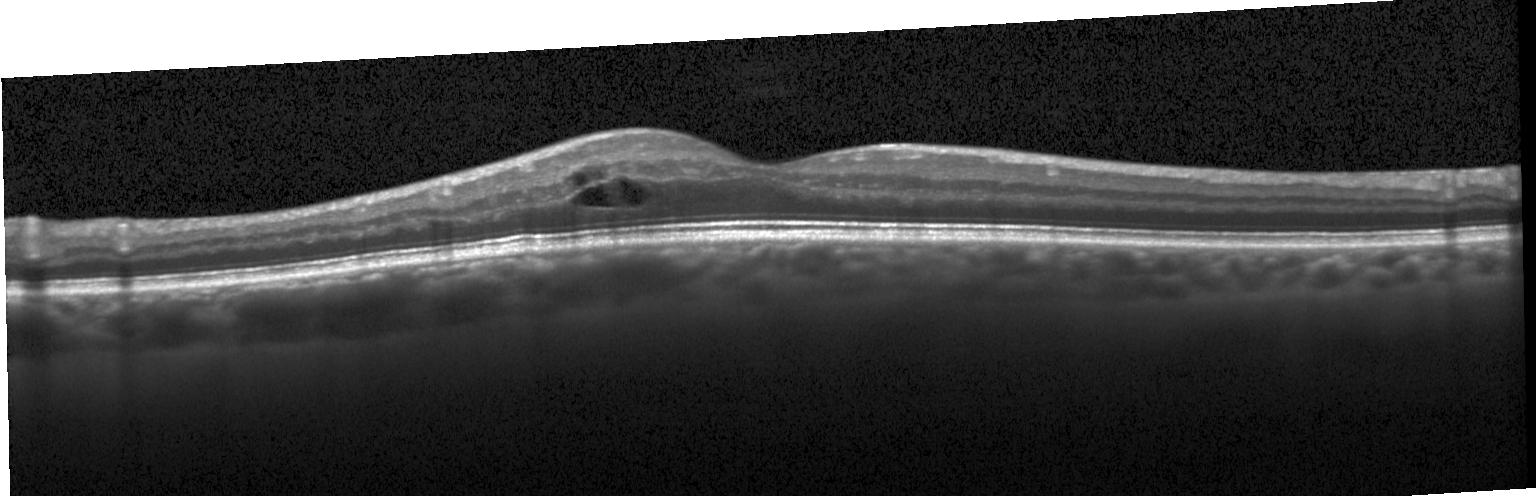
Through the macula; retinal OCT cross-section
Macular OCT: diabetic macular edema.